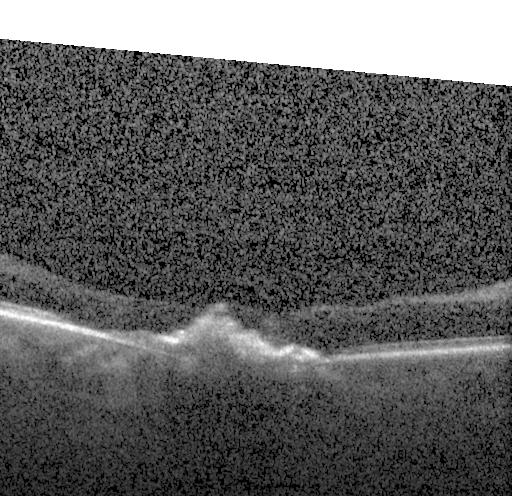

OCT scan showing a choroidal neovascular membrane.